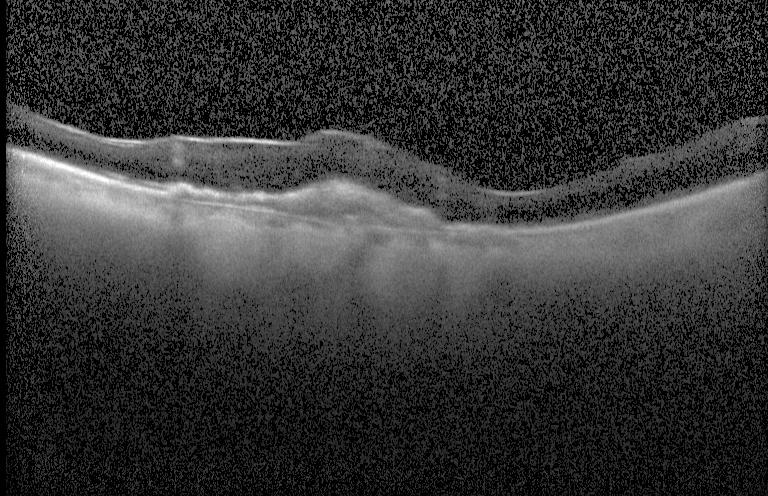
Retinal OCT B-scan — The scan shows choroidal neovascularization.